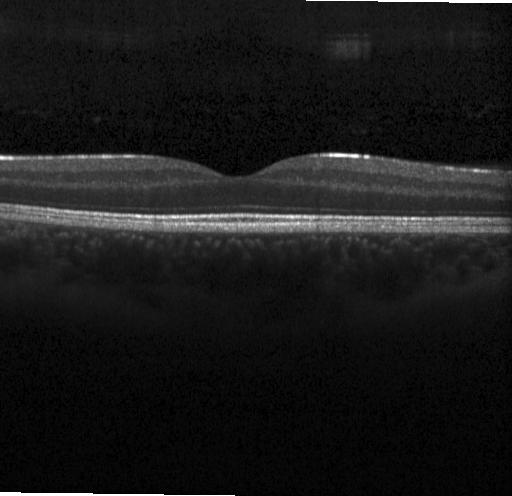
OCT B-scan
Assessment: no choroidal neovascularization, no diabetic macular edema, and no drusen.